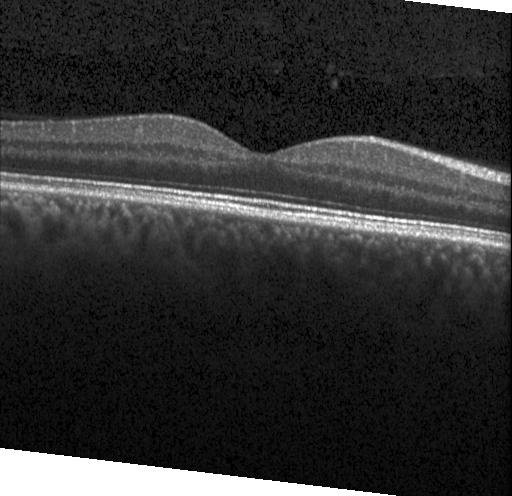 Impression: no evidence of choroidal neovascularization, diabetic macular edema, or drusen.